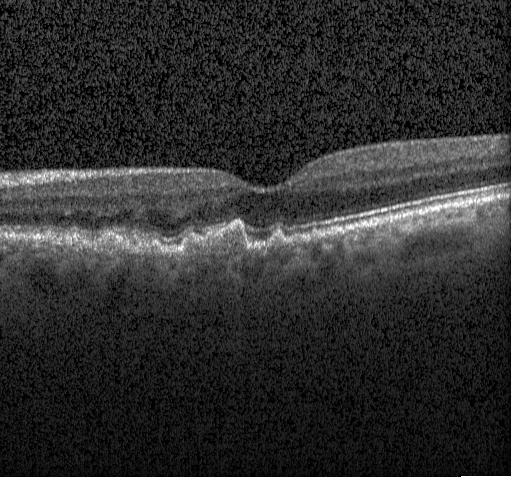 OCT finding: drusen.